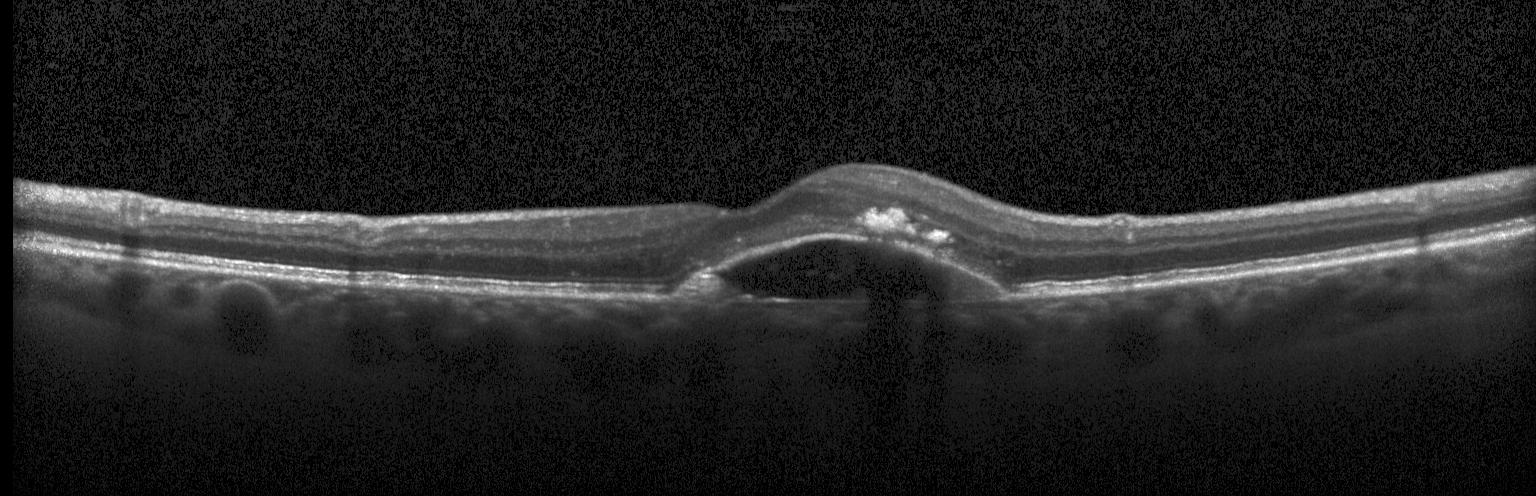

Spectral-domain optical coherence tomography, retinal OCT B-scan.
A choroidal neovascular membrane.